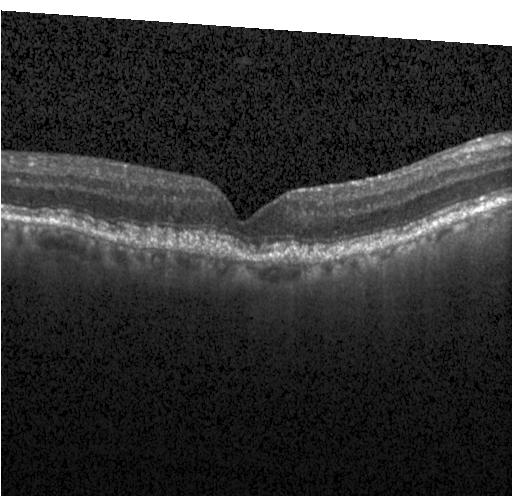
Diagnosis: drusen.